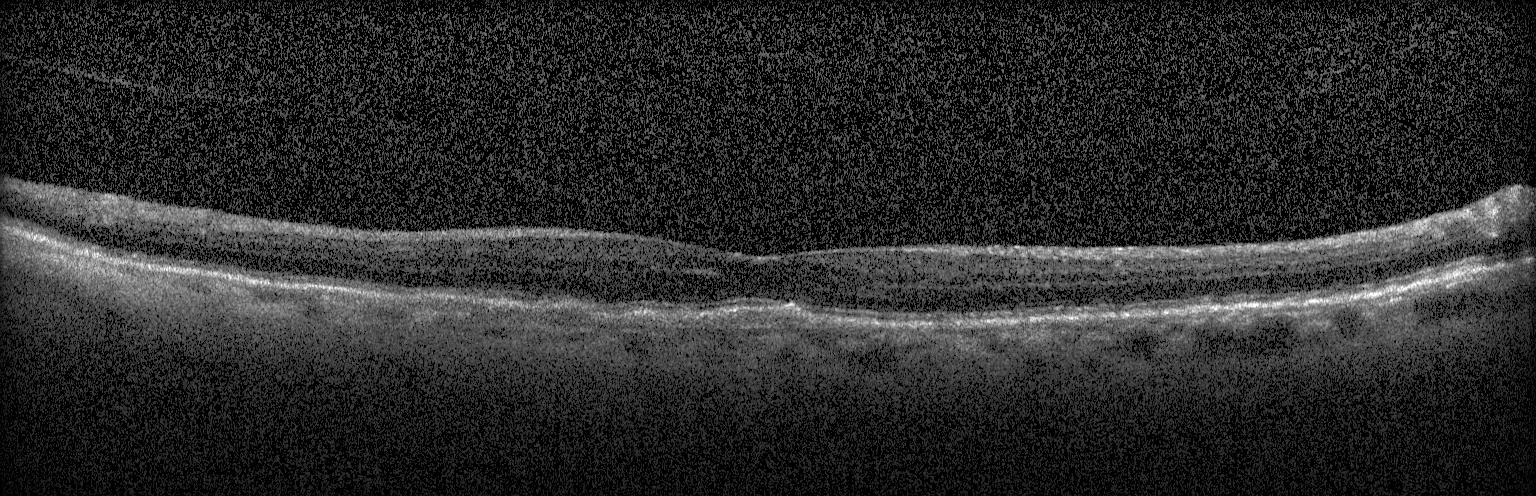

Retinal OCT cross-section
The scan shows a choroidal neovascular membrane.